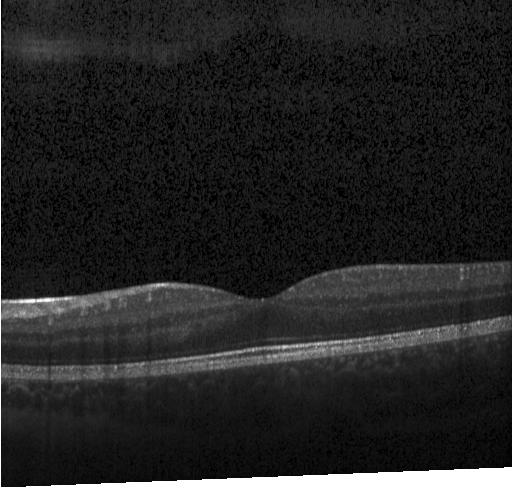

Assessment: no evidence of choroidal neovascularization, diabetic macular edema, or drusen.